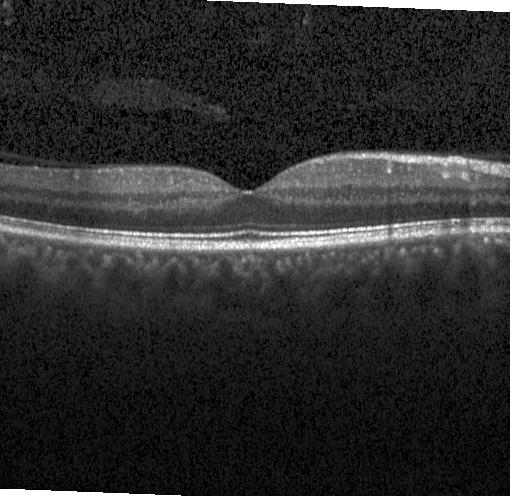 Dx: no choroidal neovascularization, no diabetic macular edema, and no drusen.